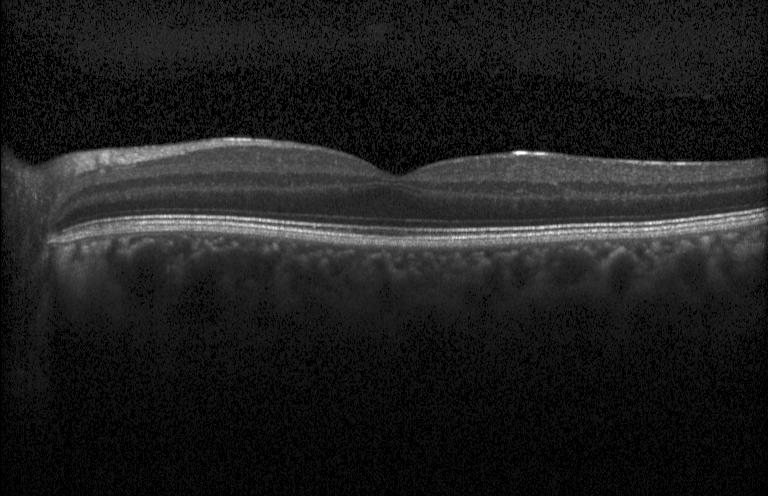
Neither CNV, DME, nor drusen.